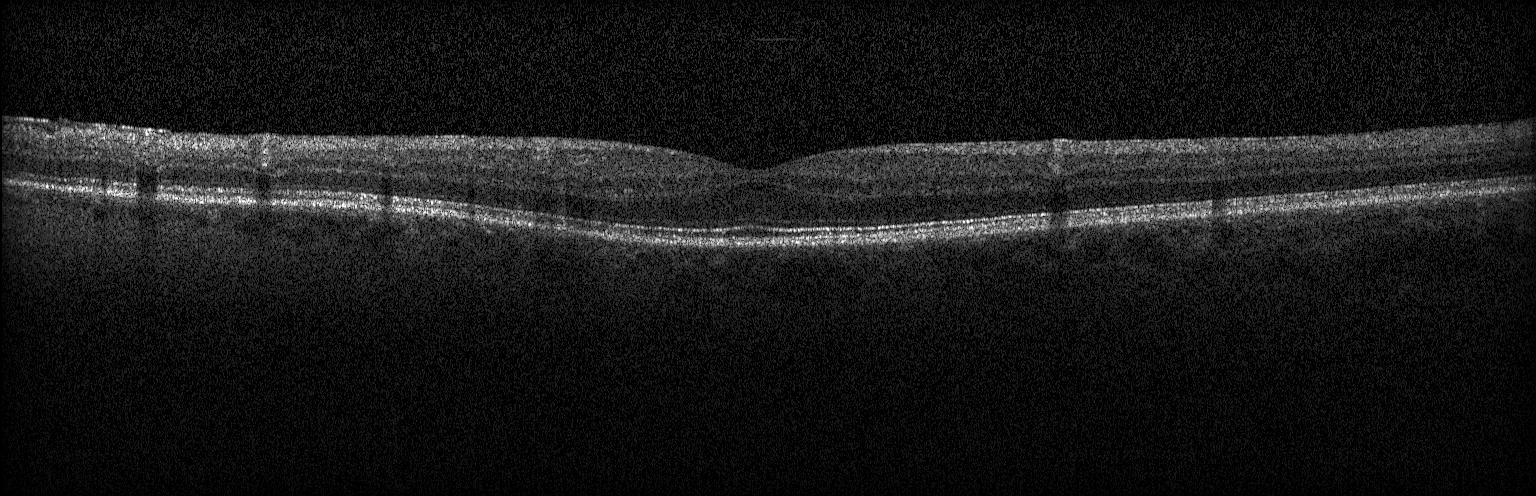

Optical coherence tomography scan, centered on the fovea. This B-scan demonstrates neither choroidal neovascularization, diabetic macular edema, nor drusen.